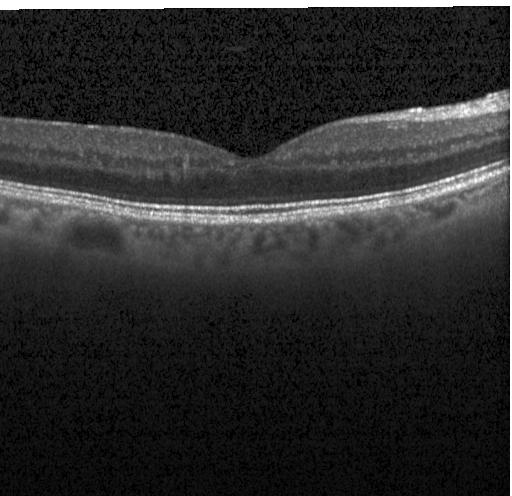 OCT B-scan.
Diagnosis: no choroidal neovascularization, no diabetic macular edema, and no drusen.